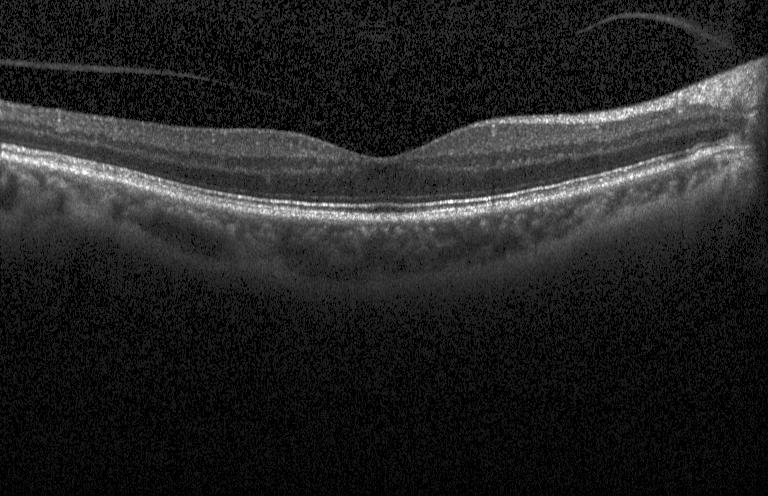 Optical coherence tomography B-scan. Dx: no choroidal neovascularization, diabetic macular edema, or drusen.